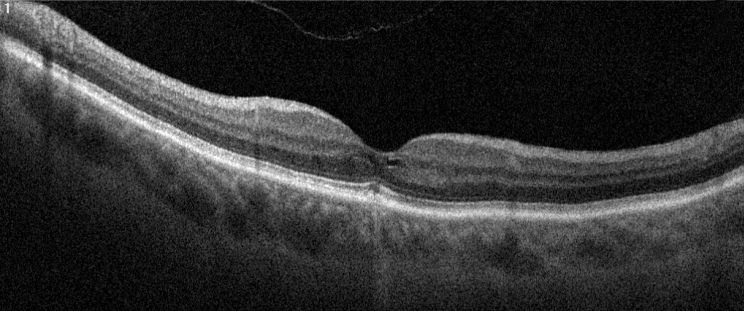

Retinal OCT cross-section showing AMD.